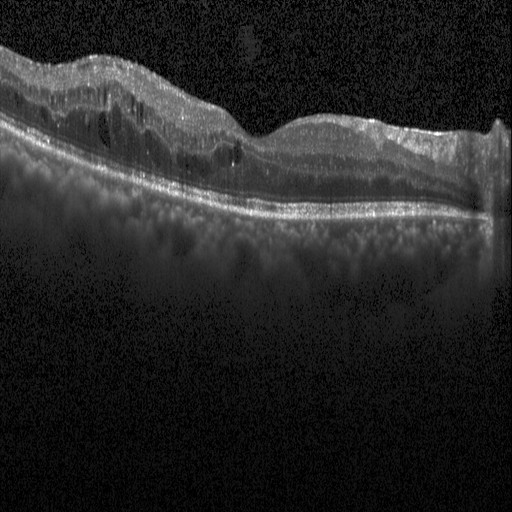

Optical coherence tomography scan; Heidelberg Spectralis OCT system; macular scan; SD-OCT
DME.